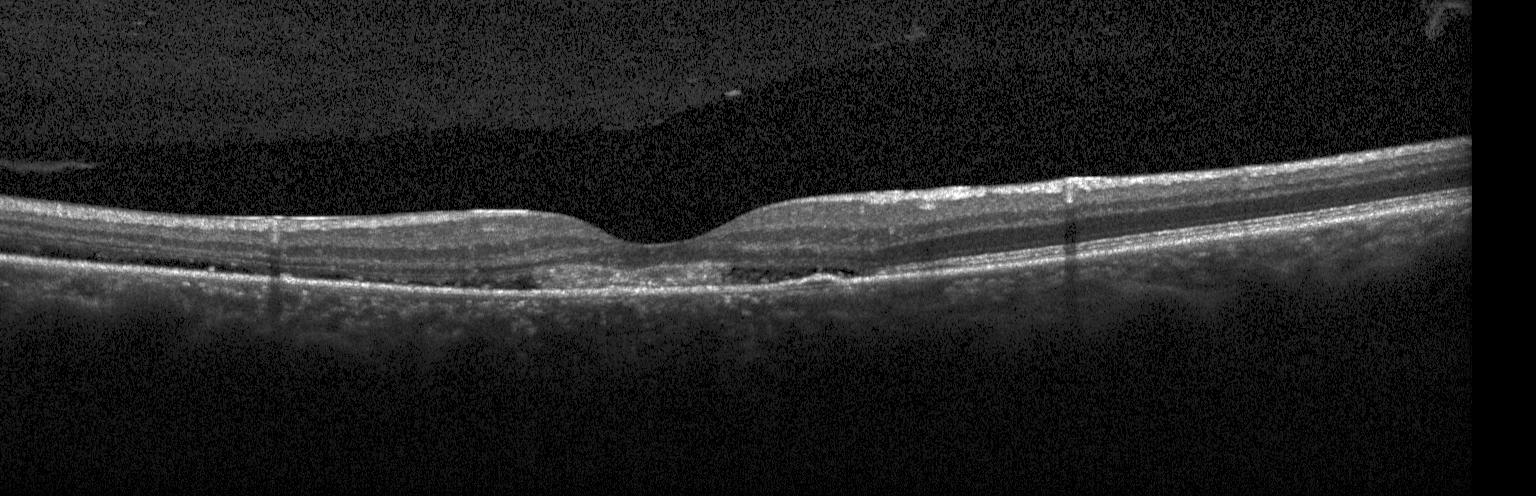 Through the macula · retinal OCT cross-section · spectral-domain OCT · Heidelberg Spectralis
The scan shows a choroidal neovascular membrane.